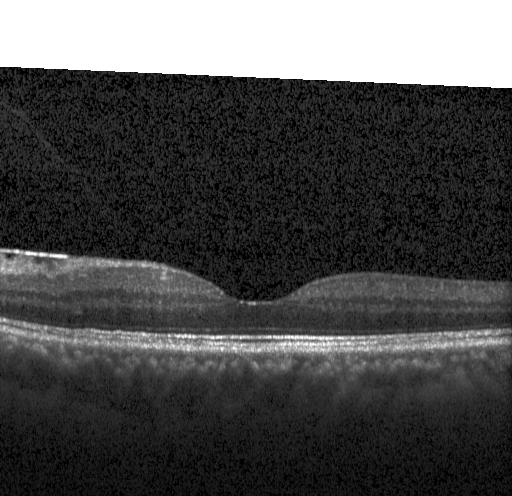

OCT line scan. Finding: no CNV, DME, or drusen.